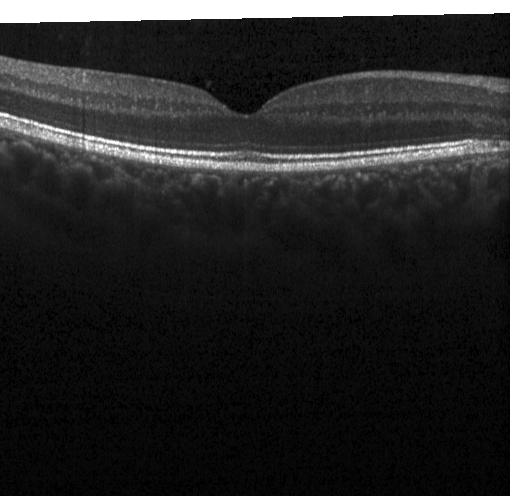
Acquired on a Heidelberg Spectralis · optical coherence tomography B-scan · SD-OCT · horizontal scan through the fovea
Assessment: no CNV, no DME, and no drusen.